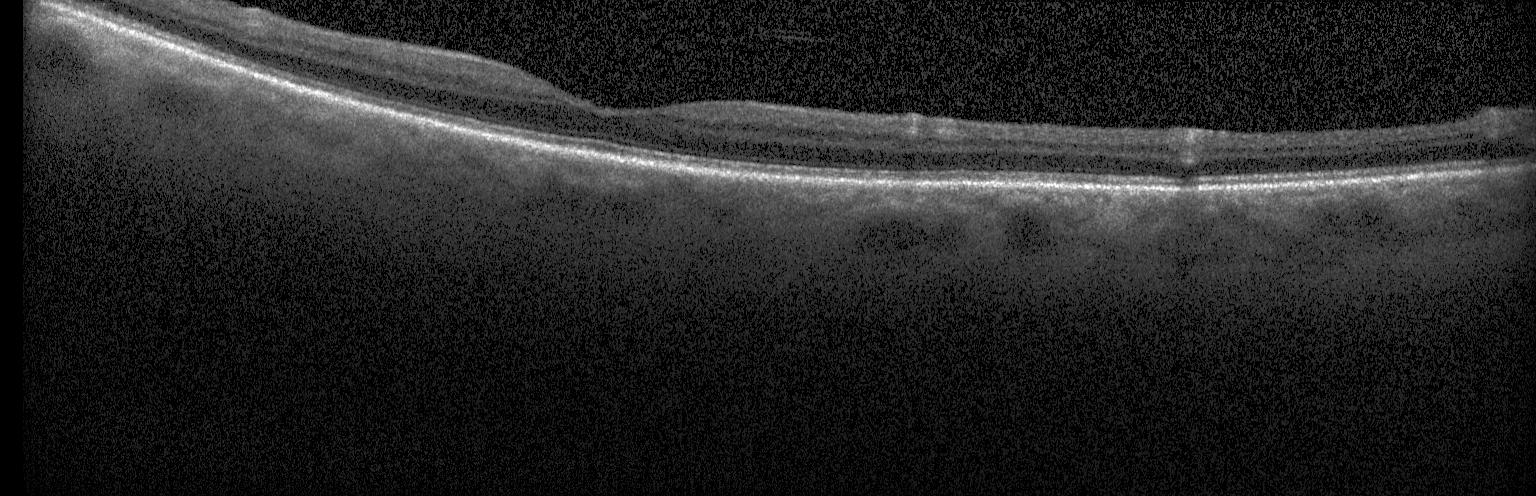 Finding: no evidence of choroidal neovascularization, diabetic macular edema, or drusen.